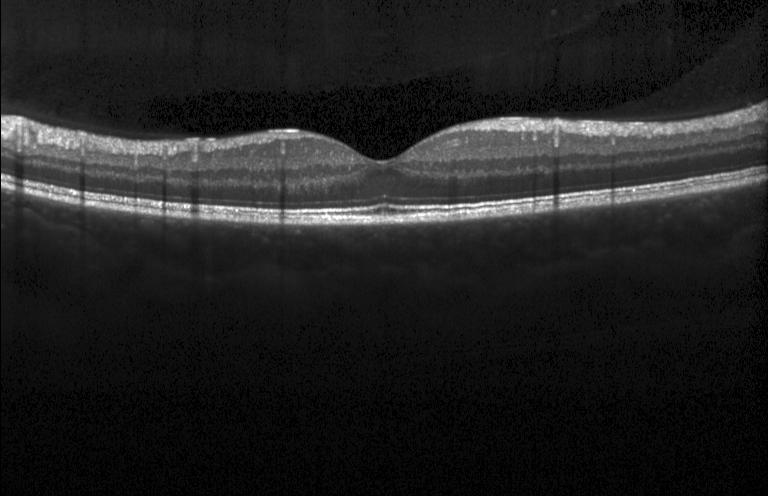
Retinal OCT cross-section; acquired on a Heidelberg Spectralis.
The scan shows no choroidal neovascularization, no diabetic macular edema, and no drusen.